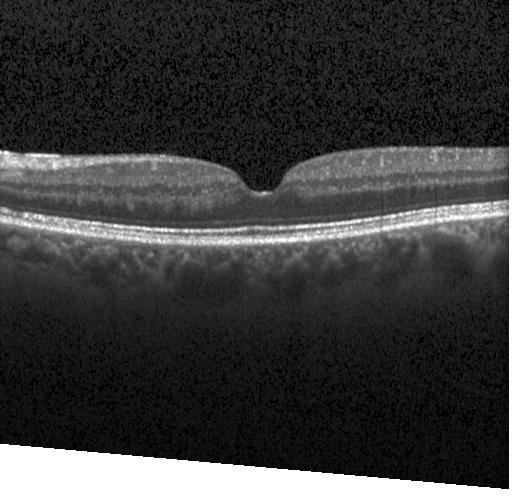

Macular scan. Optical coherence tomography B-scan. Heidelberg Spectralis — Dx: no evidence of choroidal neovascularization, diabetic macular edema, or drusen.